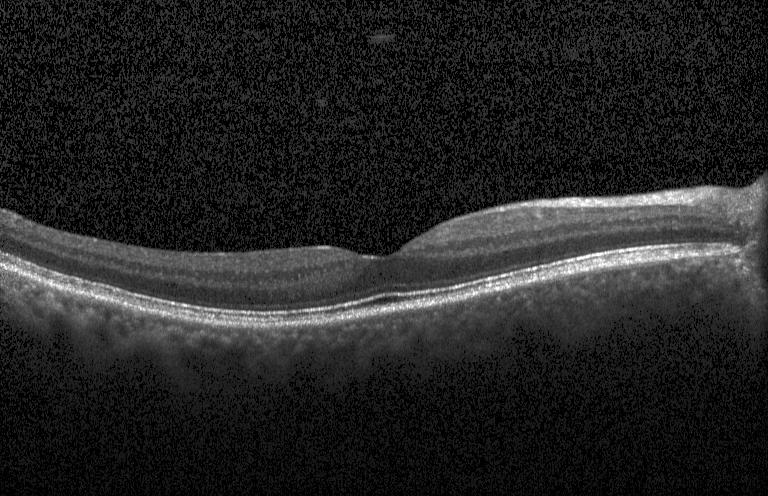

SD-OCT. Macular scan. Heidelberg Spectralis OCT system. Retinal OCT B-scan. Assessment: neither choroidal neovascularization, diabetic macular edema, nor drusen.